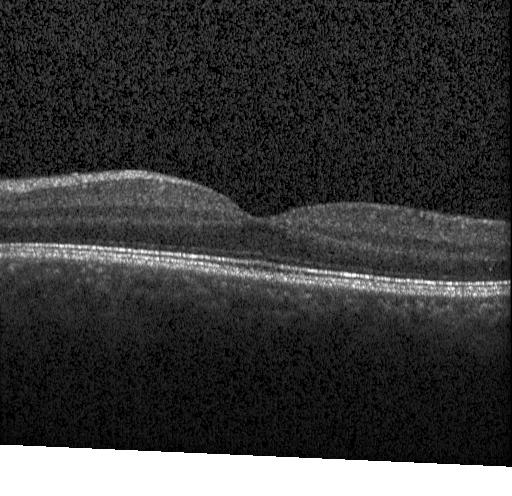
Fovea-centered. Optical coherence tomography B-scan. Heidelberg Spectralis OCT system.
This B-scan demonstrates neither choroidal neovascularization, diabetic macular edema, nor drusen.